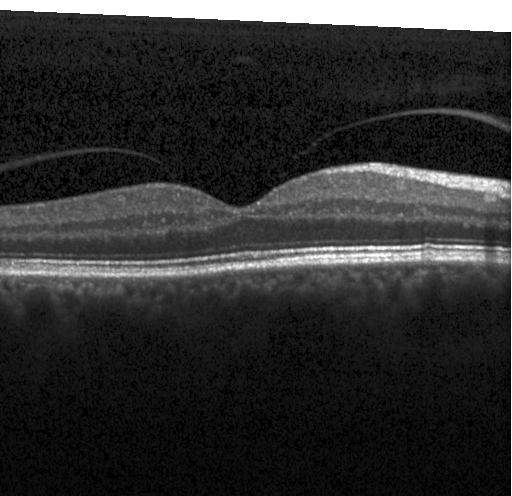
SD-OCT, retinal OCT cross-section.
Impression: no CNV, DME, or drusen.